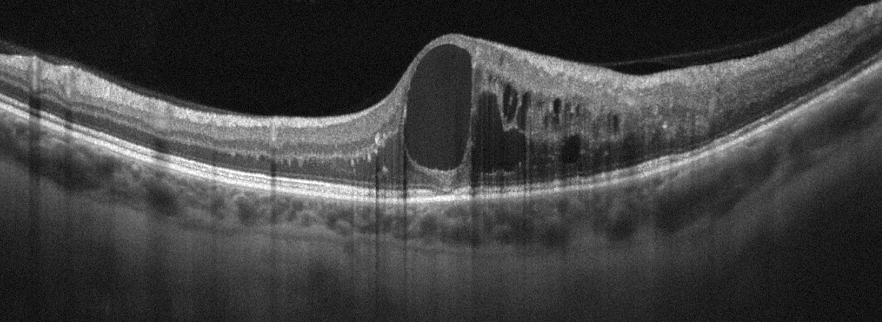 Optovue Avanti RTVue XR; OCT line scan.
Finding: retinal vein occlusion (RVO).